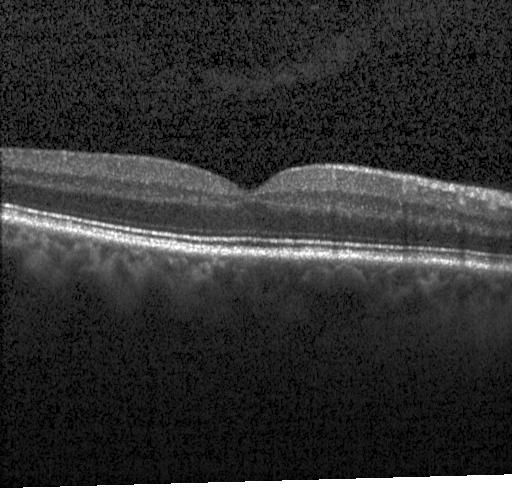

Retinal OCT B-scan; spectral-domain OCT — Impression: no choroidal neovascularization, no diabetic macular edema, and no drusen.